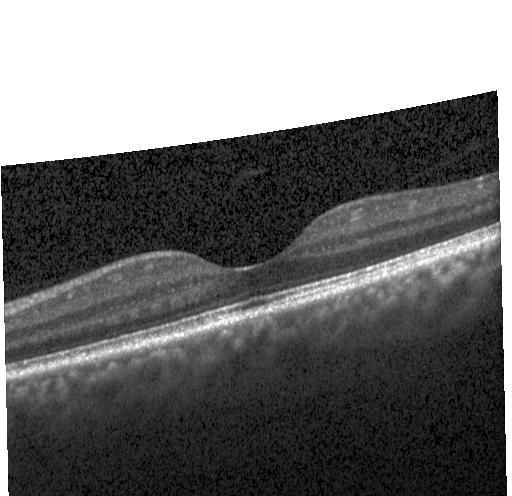

Retinal OCT B-scan — Finding: no choroidal neovascularization, no diabetic macular edema, and no drusen.